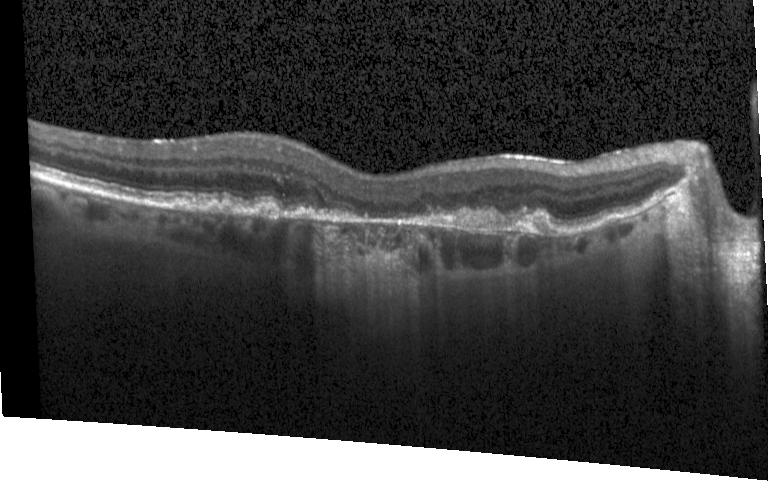
Macular OCT: a choroidal neovascular membrane.